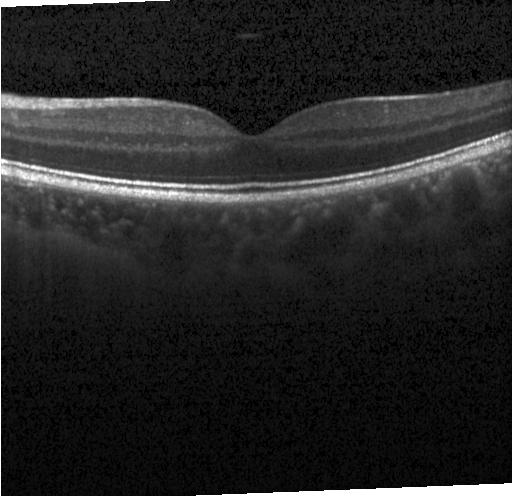

OCT B-scan. Fovea-centered. SD-OCT
Finding: no evidence of choroidal neovascularization, diabetic macular edema, or drusen.